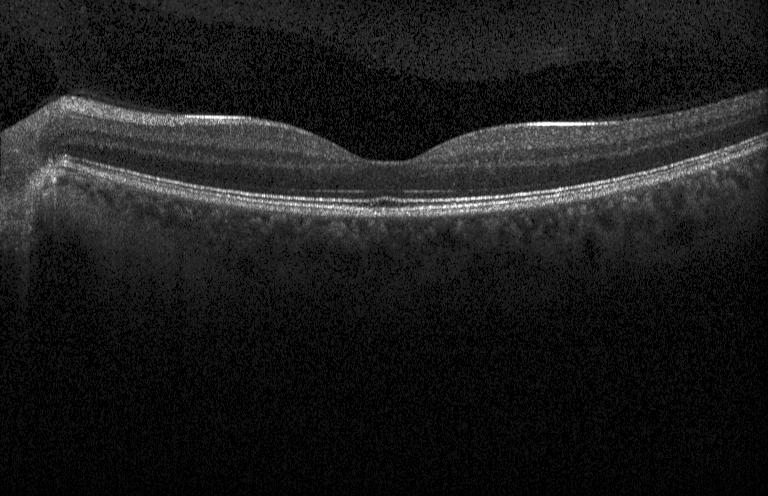

Dx: neither choroidal neovascularization, diabetic macular edema, nor drusen.